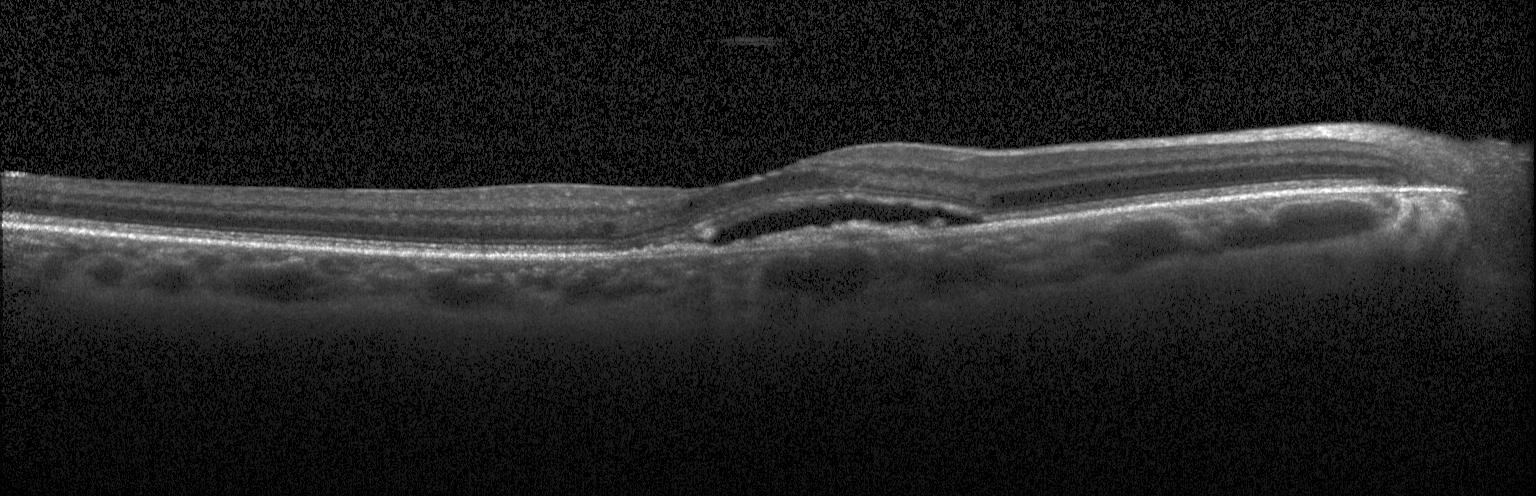 OCT B-scan
Impression: a choroidal neovascular membrane.